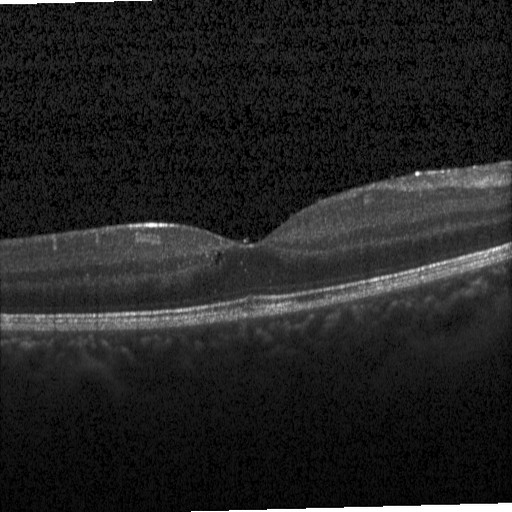 Heidelberg Spectralis, spectral-domain OCT, OCT line scan, horizontal scan through the fovea.
Assessment: diabetic macular edema (DME).